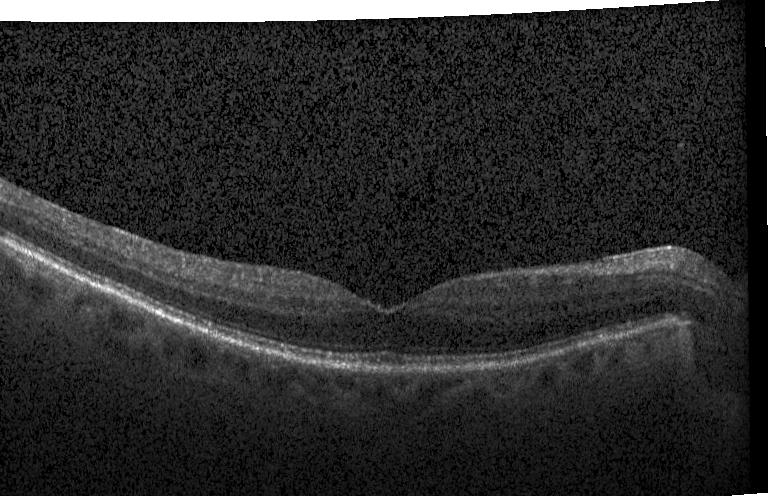 SD-OCT, instrument: Heidelberg Spectralis, OCT B-scan — Dx: no evidence of choroidal neovascularization, diabetic macular edema, or drusen.